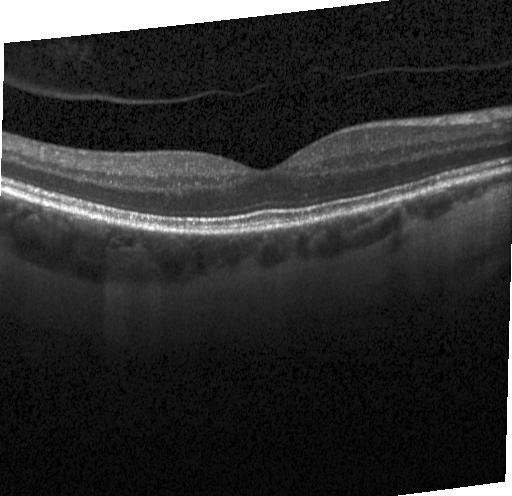
Spectral-domain OCT; Heidelberg Spectralis; fovea-centered; OCT B-scan — Dx: neither CNV, DME, nor drusen.